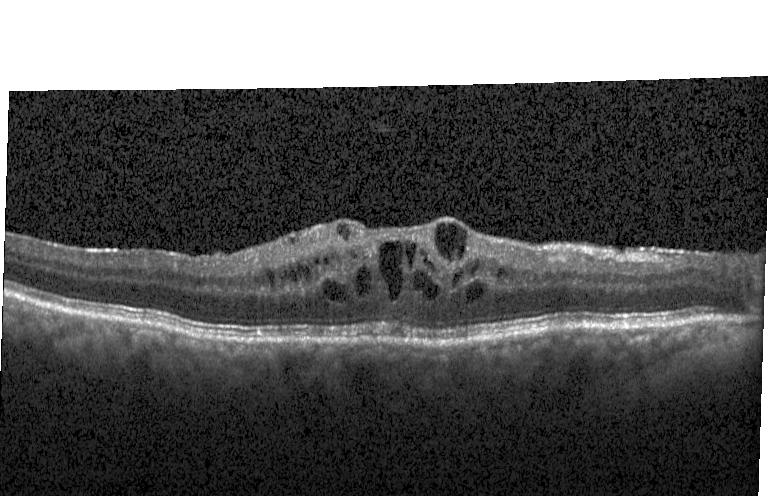

Optical coherence tomography B-scan · macular scan · acquired on a Heidelberg Spectralis
Diagnosis: diabetic macular edema.